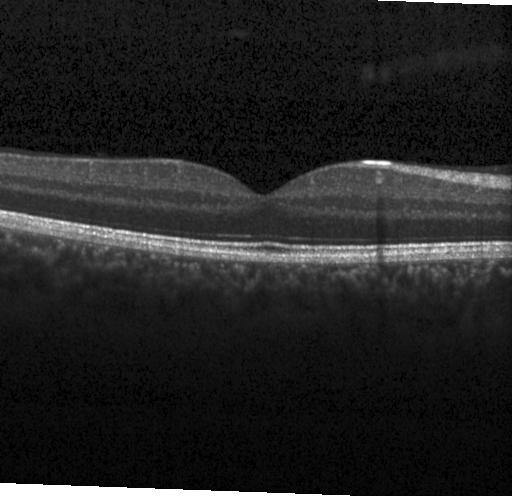

Assessment: no choroidal neovascularization, diabetic macular edema, or drusen.